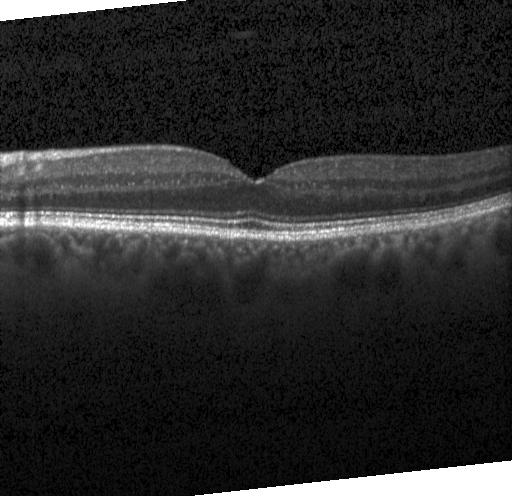 Optical coherence tomography scan; Heidelberg Spectralis; SD-OCT; horizontal scan through the fovea
Impression: no choroidal neovascularization, no diabetic macular edema, and no drusen.